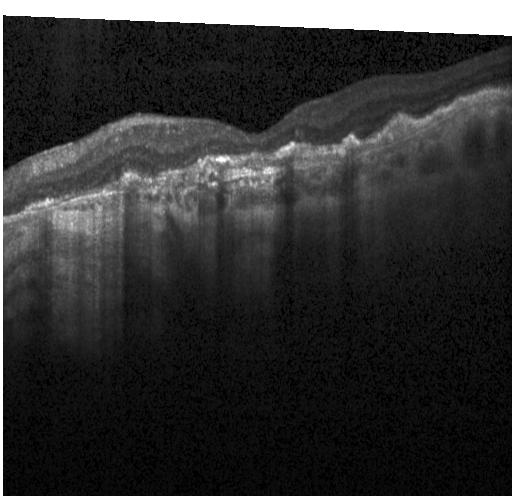
Retinal OCT cross-section.
Macular OCT: a choroidal neovascular membrane.